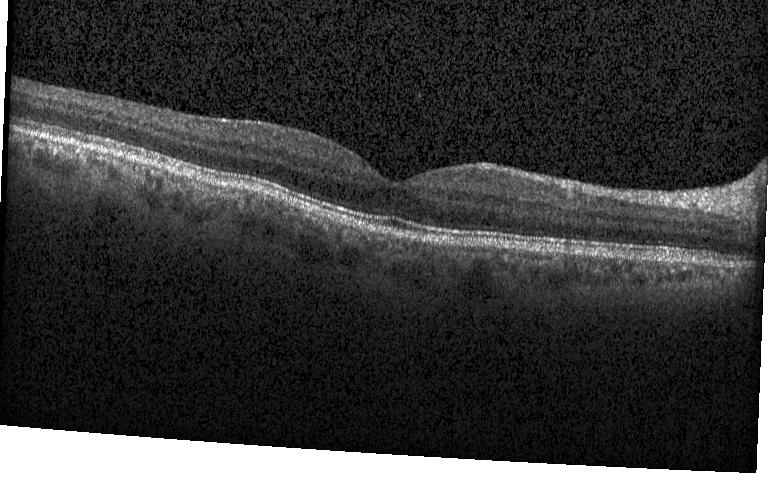

Spectral-domain OCT; optical coherence tomography scan; instrument: Heidelberg Spectralis
Diagnosis: no CNV, no DME, and no drusen.